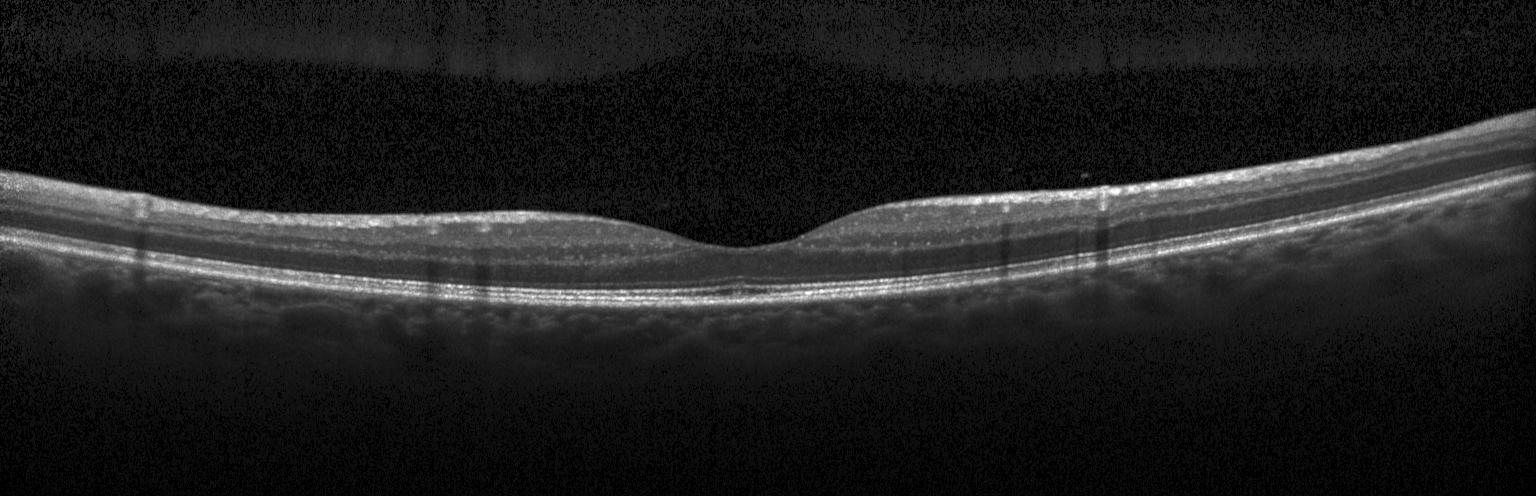 SD-OCT, OCT line scan. Assessment: neither choroidal neovascularization, diabetic macular edema, nor drusen.